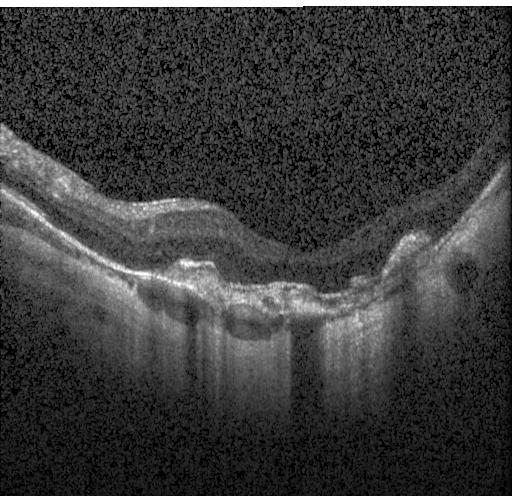
Centered on the fovea, retinal OCT cross-section, spectral-domain optical coherence tomography, instrument: Heidelberg Spectralis
Macular OCT: a choroidal neovascular membrane.